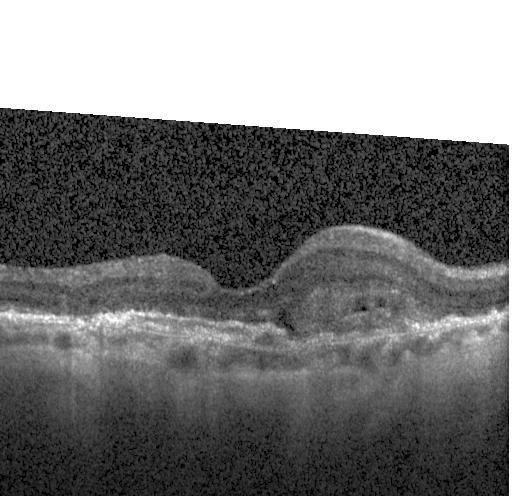 Heidelberg Spectralis; macular scan; SD-OCT; OCT line scan.
The scan shows choroidal neovascularization (CNV).